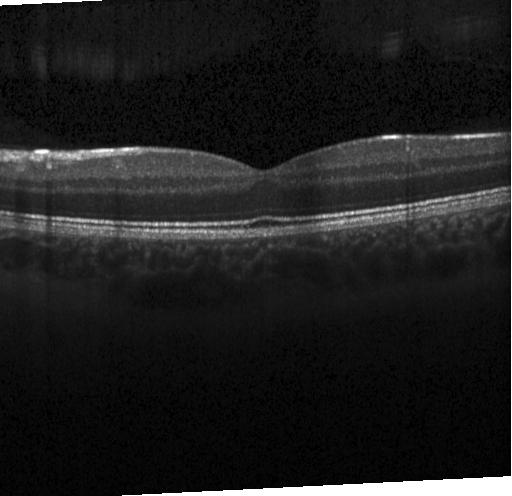
Retinal OCT cross-section — The scan shows neither choroidal neovascularization, diabetic macular edema, nor drusen.